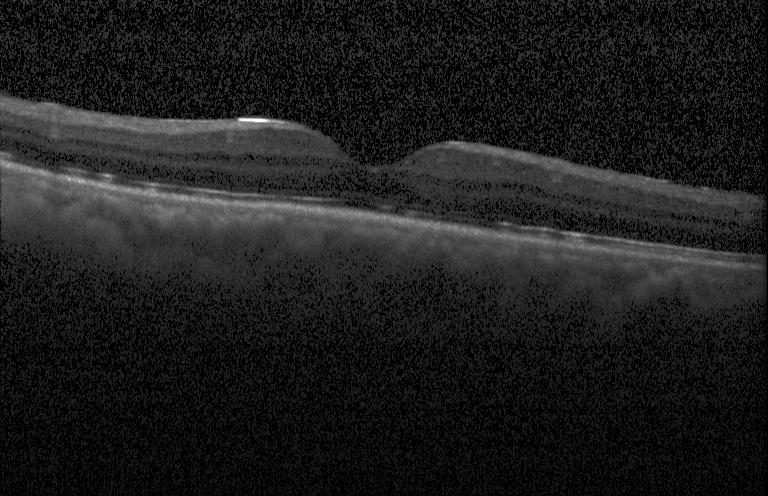 OCT scan showing no evidence of choroidal neovascularization, diabetic macular edema, or drusen.